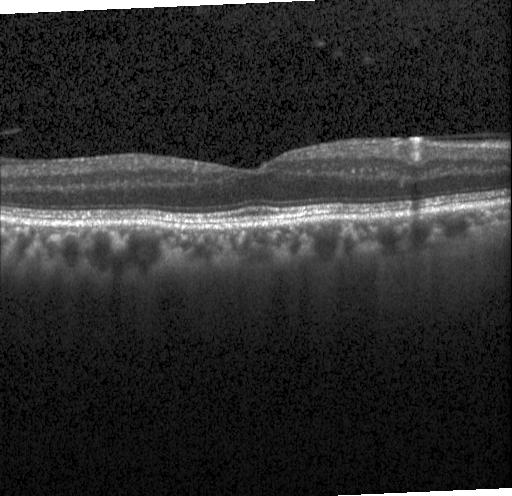

Macular OCT: neither choroidal neovascularization, diabetic macular edema, nor drusen.